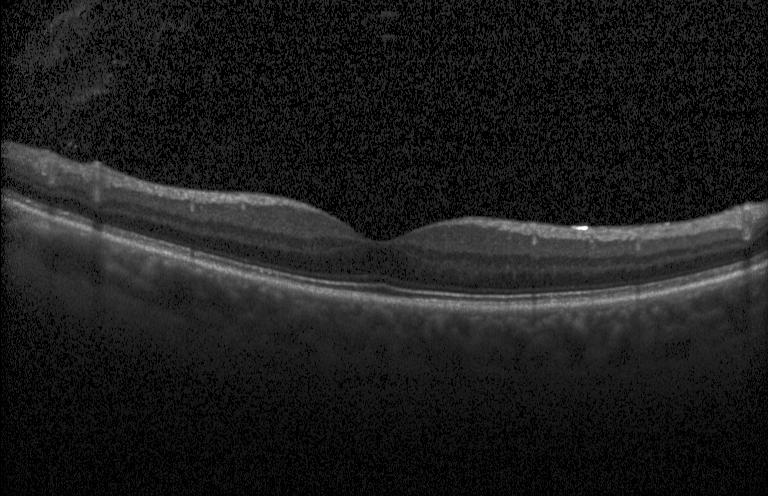
Instrument: Heidelberg Spectralis, optical coherence tomography scan, spectral-domain OCT.
Finding: neither CNV, DME, nor drusen.